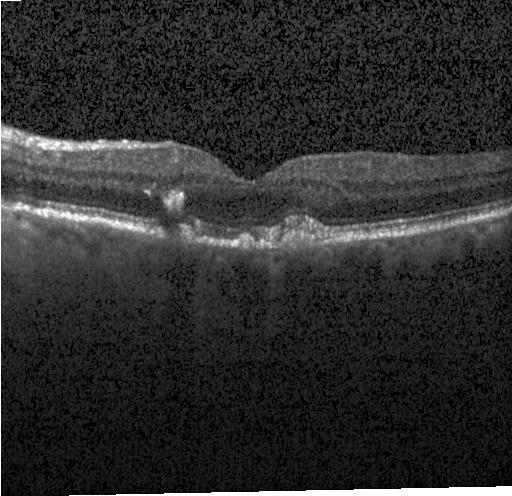 OCT scan showing sub-RPE drusenoid deposits.